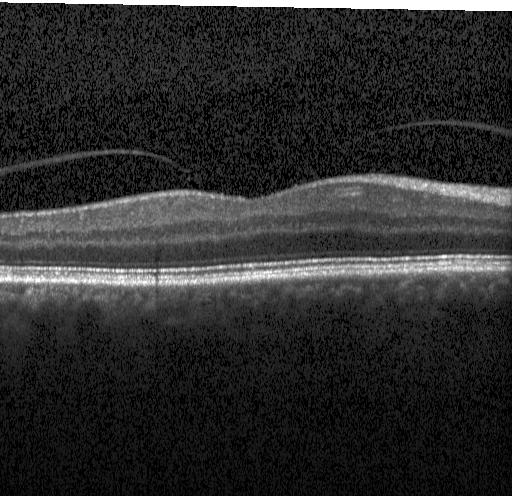 Optical coherence tomography scan, spectral-domain optical coherence tomography. Assessment: no choroidal neovascularization, no diabetic macular edema, and no drusen.